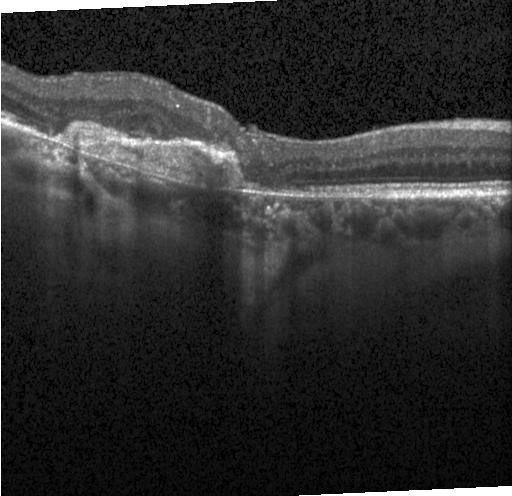

OCT finding: a choroidal neovascular membrane.